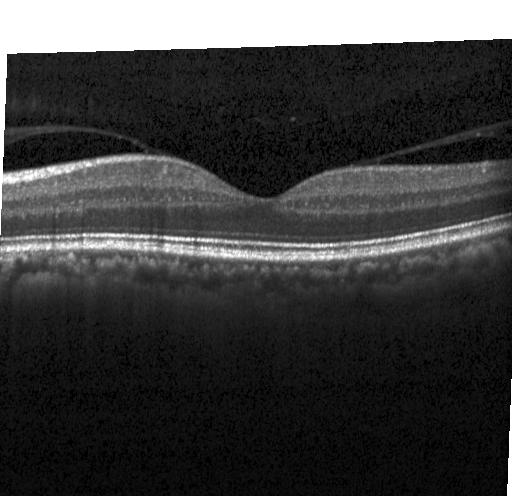

This B-scan demonstrates no evidence of CNV, DME, or drusen.